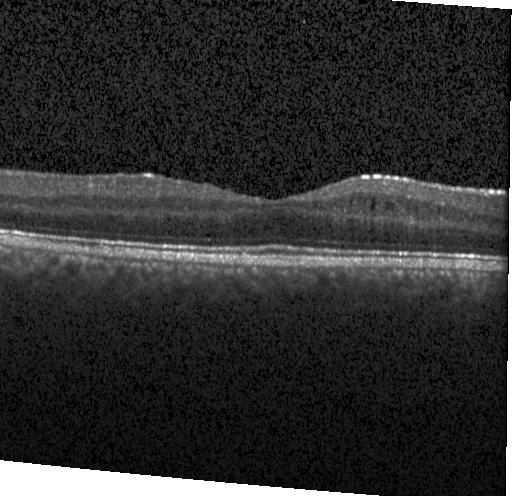

SD-OCT, optical coherence tomography scan, macular scan
OCT finding: diabetic macular edema.